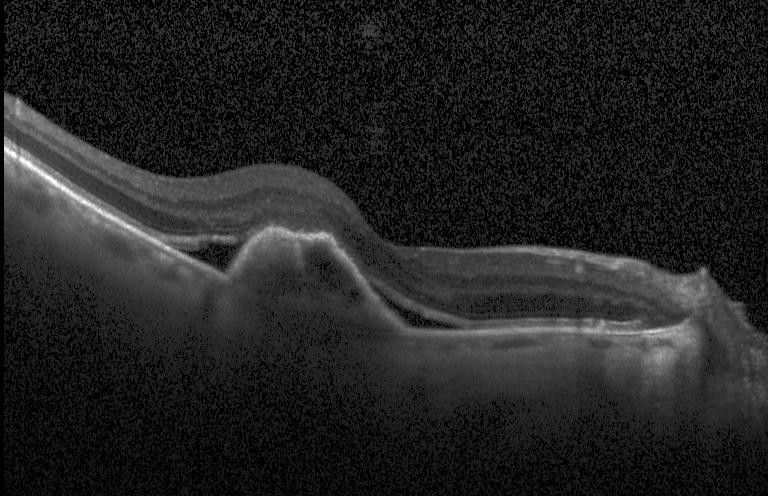

Spectral-domain optical coherence tomography; acquired on a Heidelberg Spectralis; macular scan; OCT B-scan.
Macular OCT: CNV.